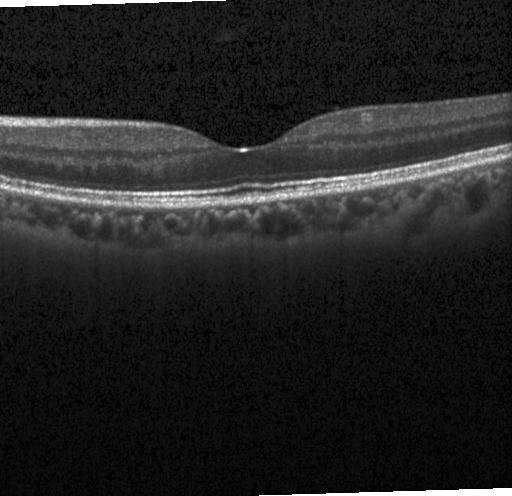
Macular OCT demonstrating no choroidal neovascularization, diabetic macular edema, or drusen.